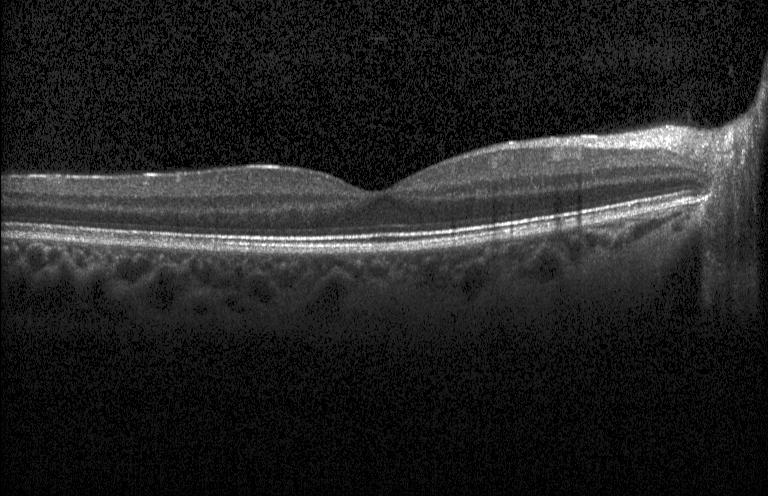

OCT B-scan showing no CNV, no DME, and no drusen.